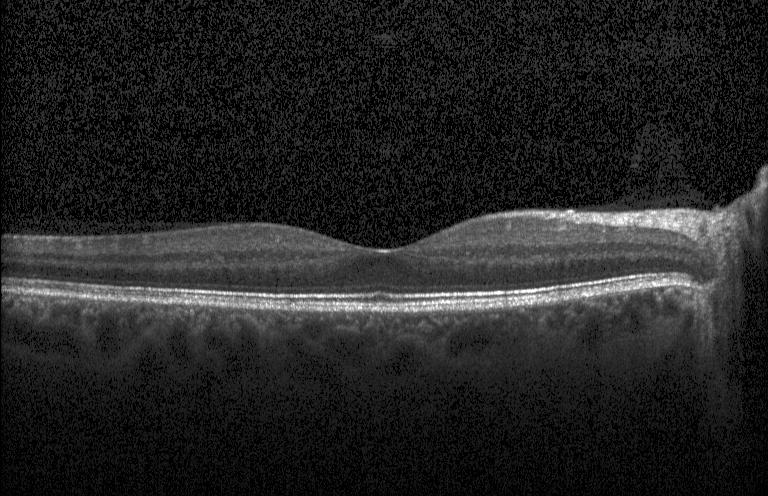 Retinal OCT cross-section. Instrument: Heidelberg Spectralis. Spectral-domain optical coherence tomography
Finding: no evidence of choroidal neovascularization, diabetic macular edema, or drusen.